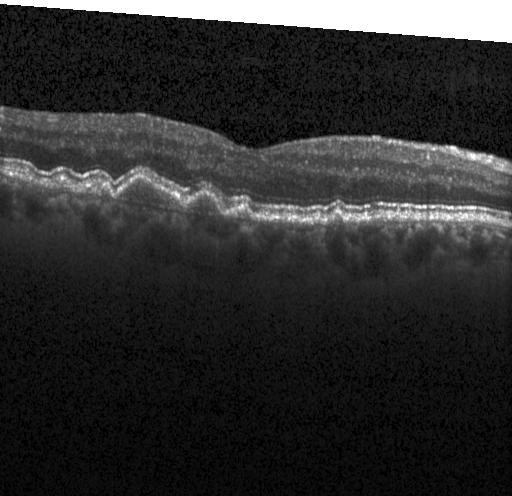 Macular OCT: multiple drusen.